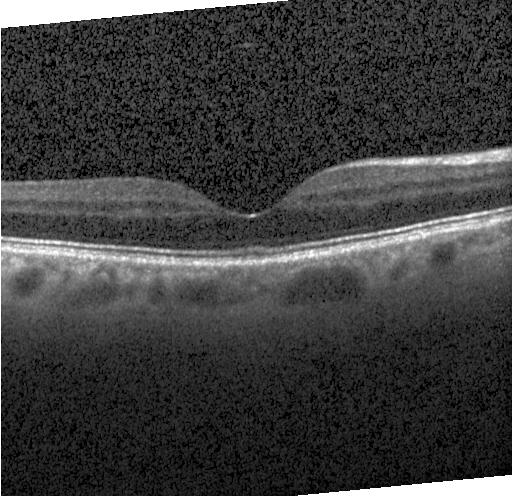 Optical coherence tomography scan
OCT finding: no CNV, no DME, and no drusen.